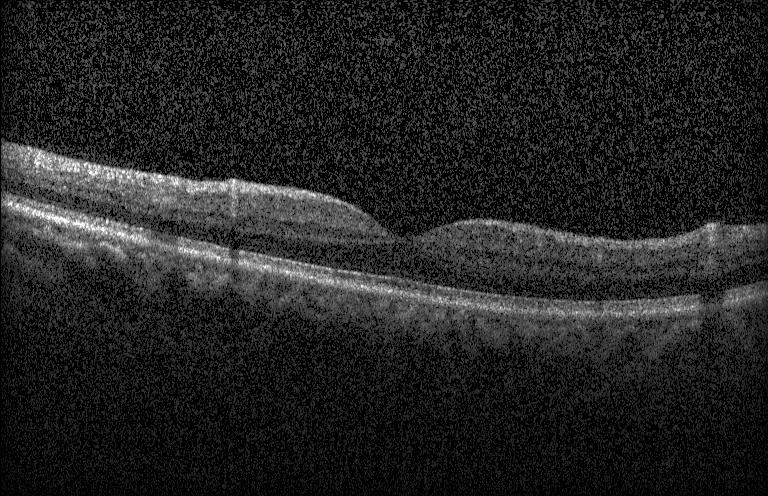

Fovea-centered. Retinal OCT B-scan. Spectral-domain optical coherence tomography
Macular OCT: no evidence of CNV, DME, or drusen.